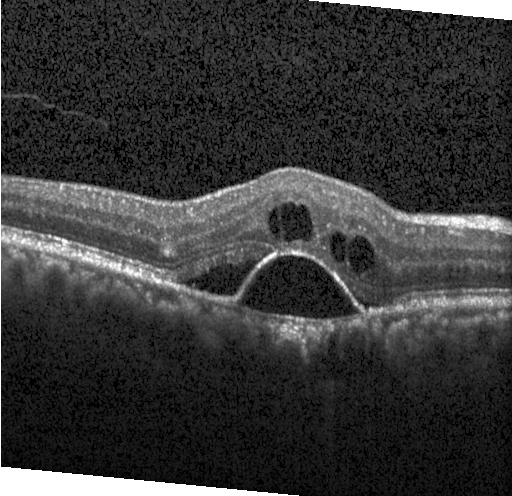
Retinal OCT cross-section showing a choroidal neovascular membrane.